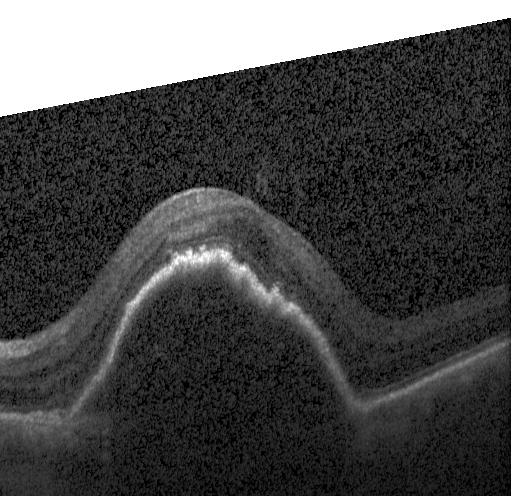
Macular OCT demonstrating a choroidal neovascular membrane.